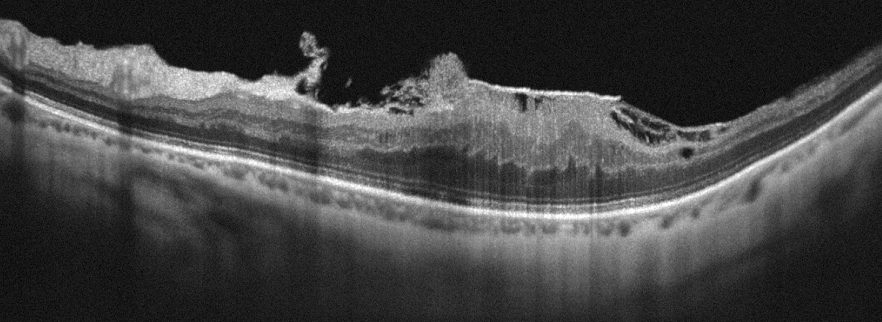 Optical coherence tomography scan, OS
Diagnosis: epiretinal membrane (ERM).